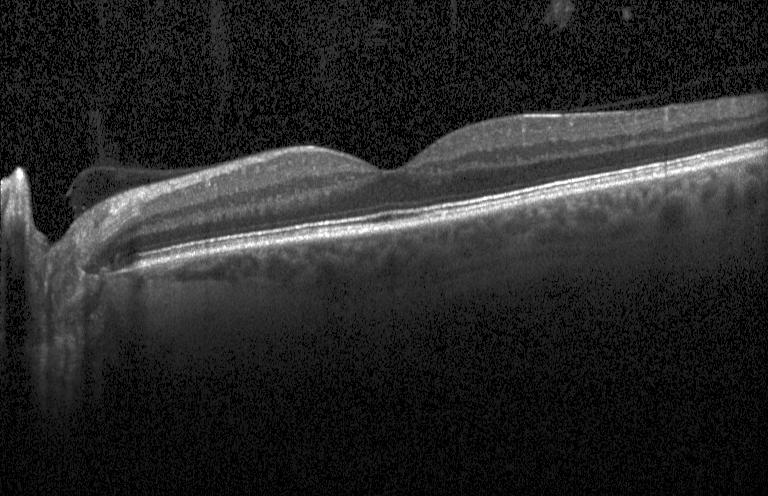

Optical coherence tomography scan. SD-OCT. Horizontal scan through the fovea — No choroidal neovascularization, no diabetic macular edema, and no drusen.